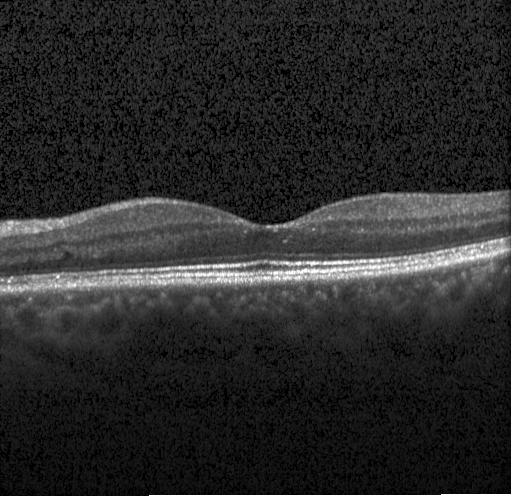
Spectral-domain optical coherence tomography. Heidelberg Spectralis OCT system. Horizontal scan through the fovea. Optical coherence tomography B-scan.
The scan shows no choroidal neovascularization, diabetic macular edema, or drusen.